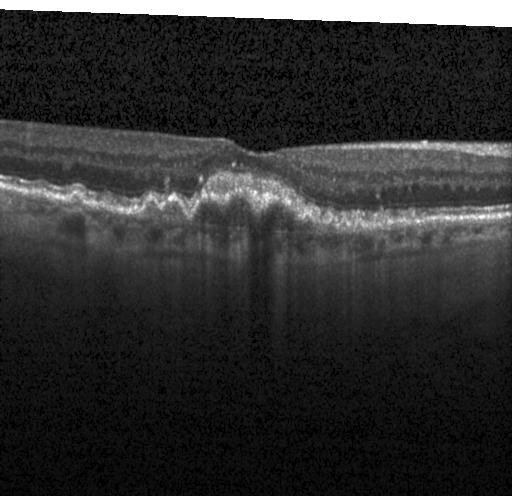 OCT line scan · centered on the fovea · SD-OCT.
Finding: a choroidal neovascular membrane.